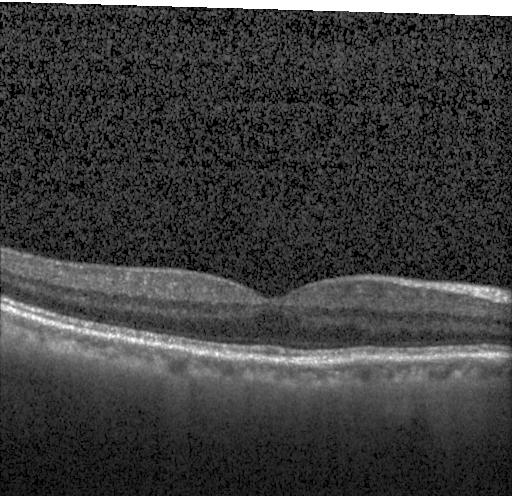

Heidelberg Spectralis OCT system. Retinal OCT B-scan. Through the macula.
The scan shows no evidence of choroidal neovascularization, diabetic macular edema, or drusen.